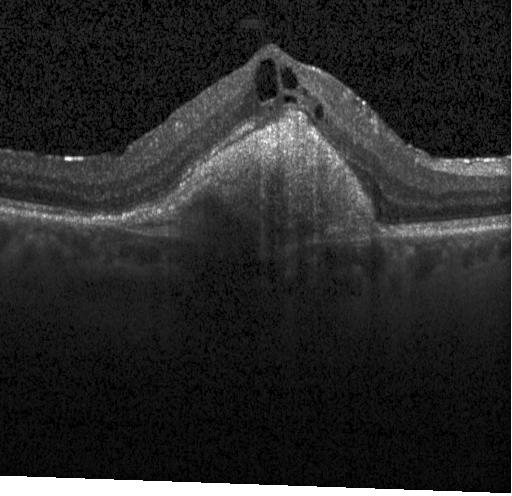 OCT B-scan. Assessment: CNV.